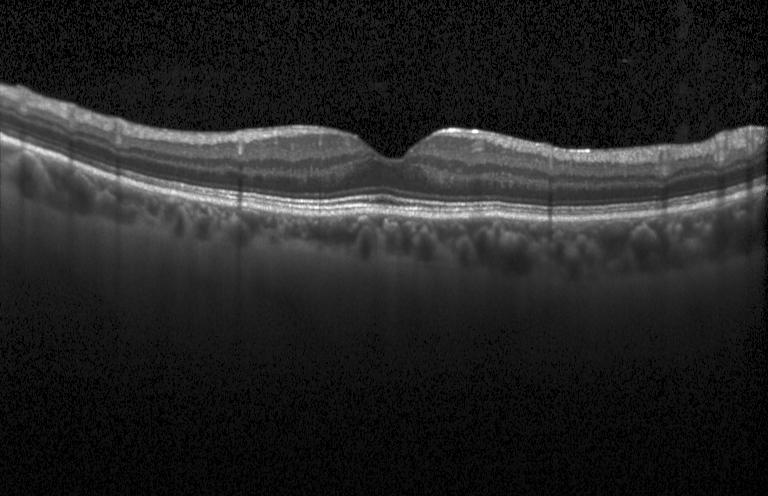
Centered on the fovea · retinal OCT cross-section. Finding: no evidence of choroidal neovascularization, diabetic macular edema, or drusen.